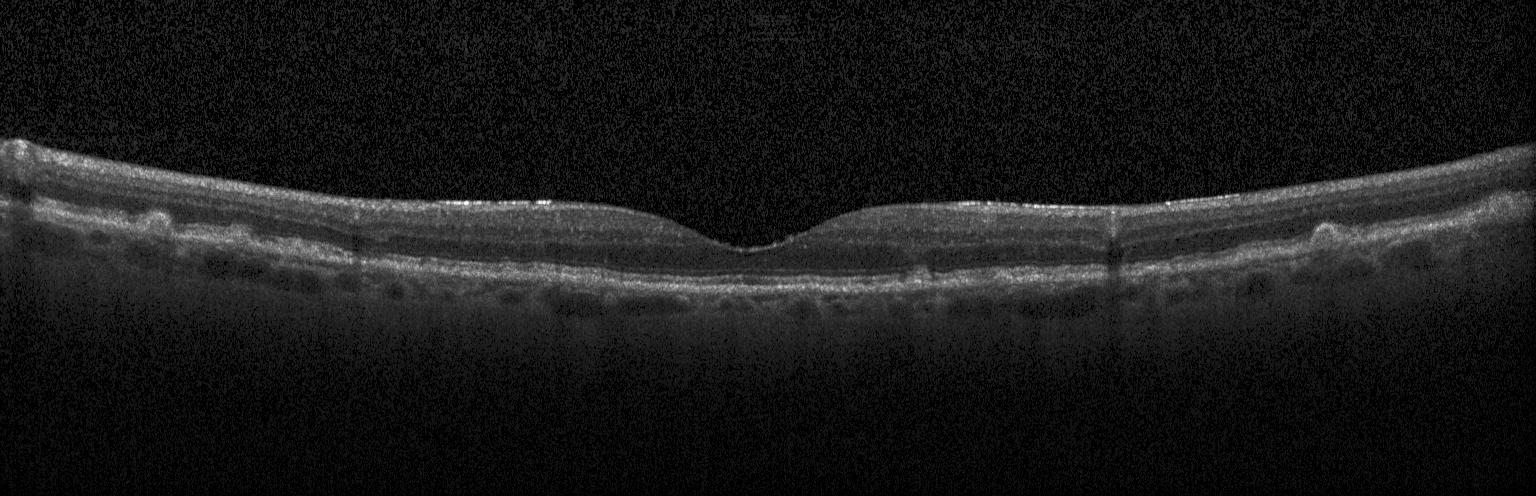 Optical coherence tomography B-scan; macular scan; spectral-domain OCT; instrument: Heidelberg Spectralis.
Impression: multiple drusen.